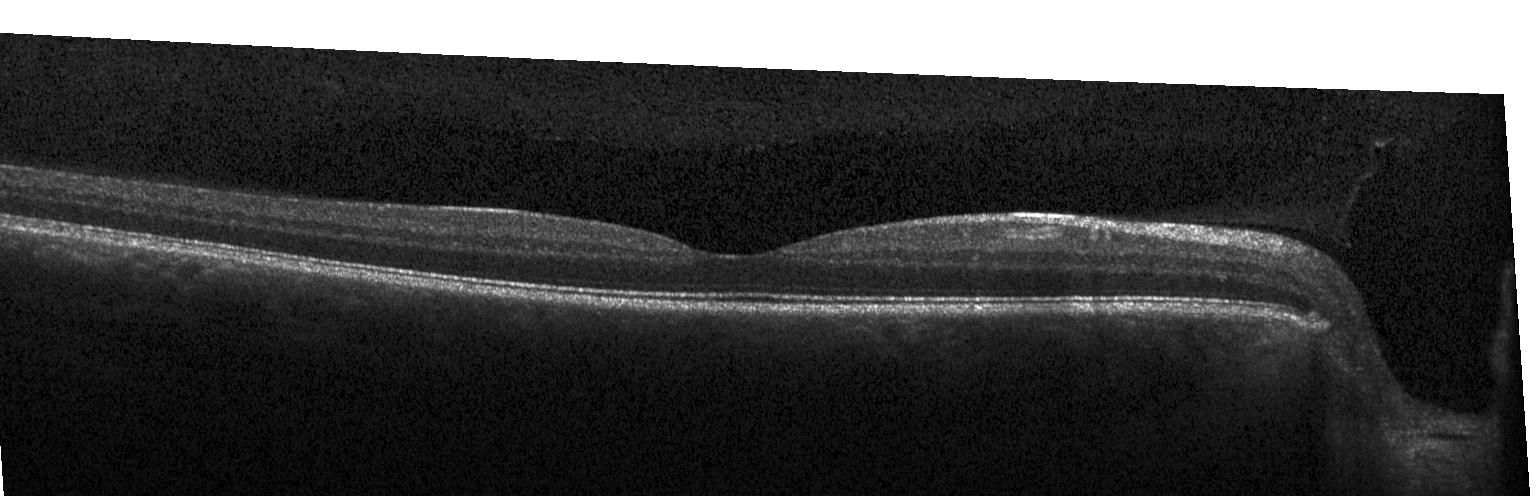 Macular OCT: neither choroidal neovascularization, diabetic macular edema, nor drusen.